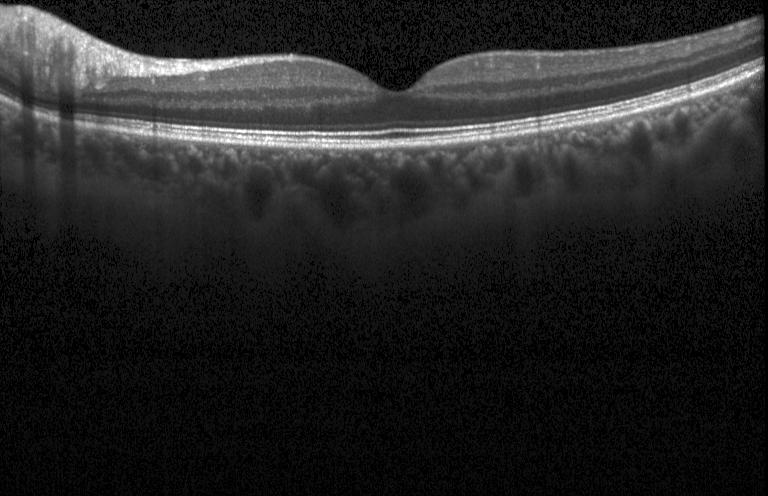 Macular OCT: no CNV, no DME, and no drusen.